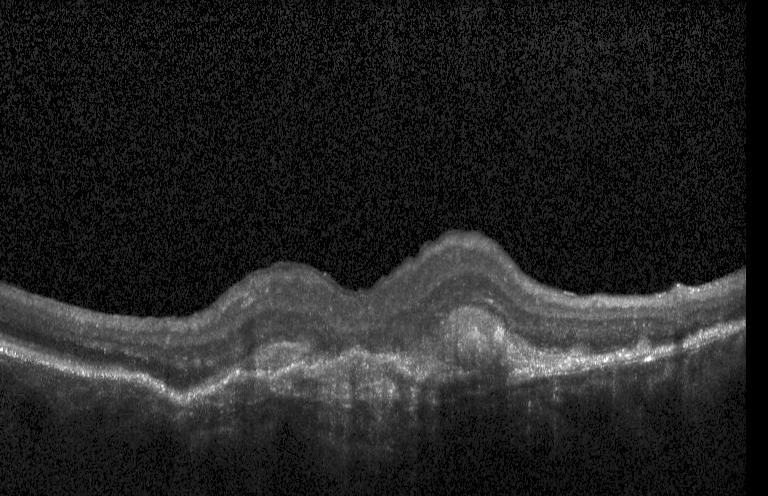
A choroidal neovascular membrane.